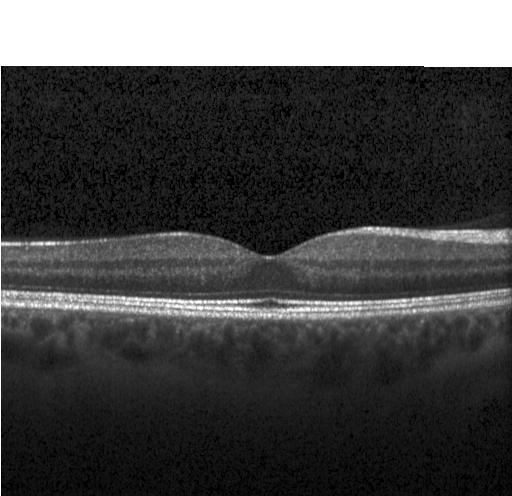 OCT line scan; spectral-domain optical coherence tomography; Heidelberg Spectralis — Neither choroidal neovascularization, diabetic macular edema, nor drusen.